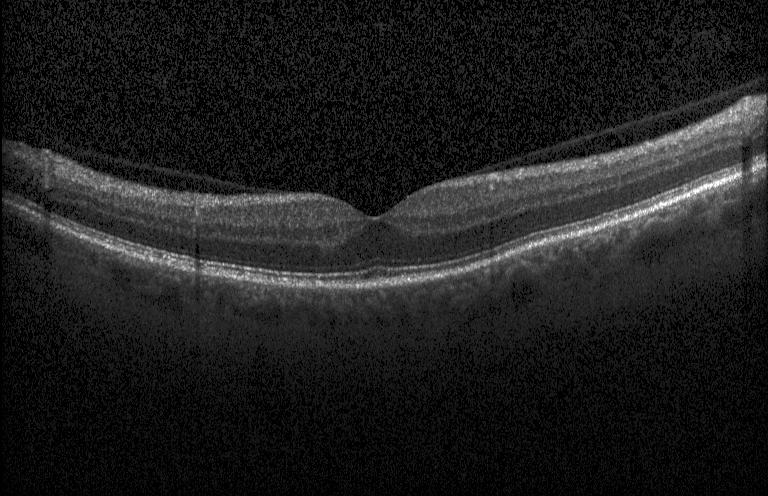 Retinal OCT cross-section showing neither choroidal neovascularization, diabetic macular edema, nor drusen.